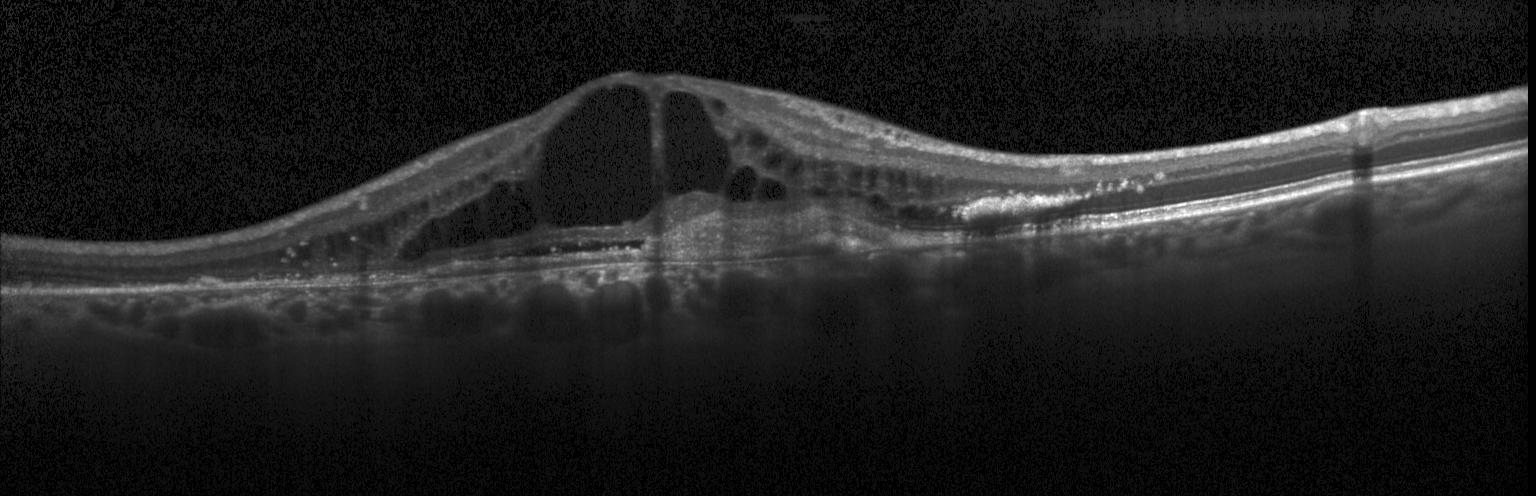 OCT finding: choroidal neovascularization.